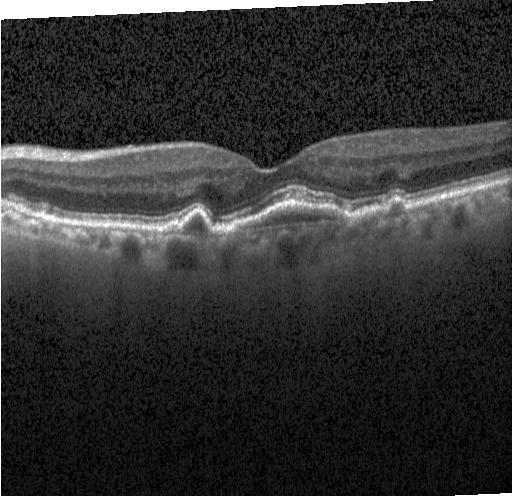
OCT B-scan. Diagnosis: a choroidal neovascular membrane.